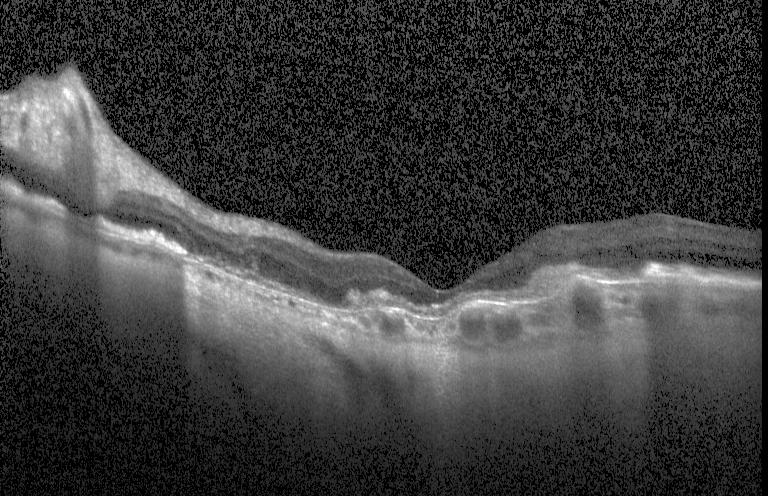

Retinal OCT cross-section. Centered on the fovea. Spectral-domain optical coherence tomography. Heidelberg Spectralis OCT system.
Finding: choroidal neovascularization.